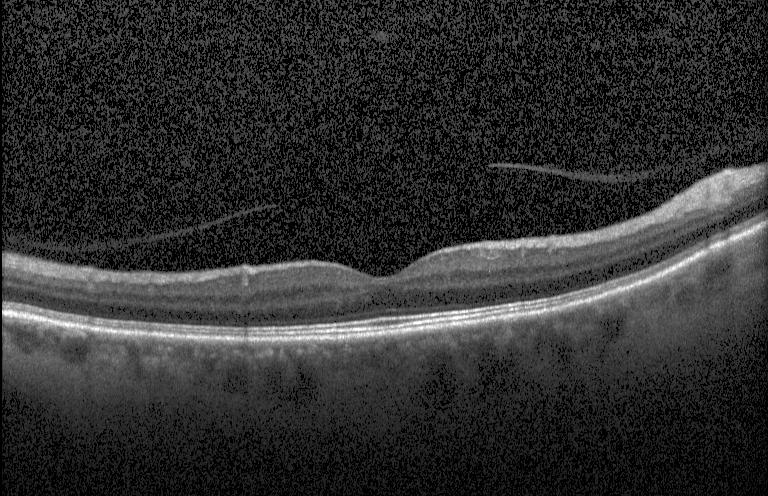

Fovea-centered. Optical coherence tomography B-scan. SD-OCT.
Impression: neither choroidal neovascularization, diabetic macular edema, nor drusen.